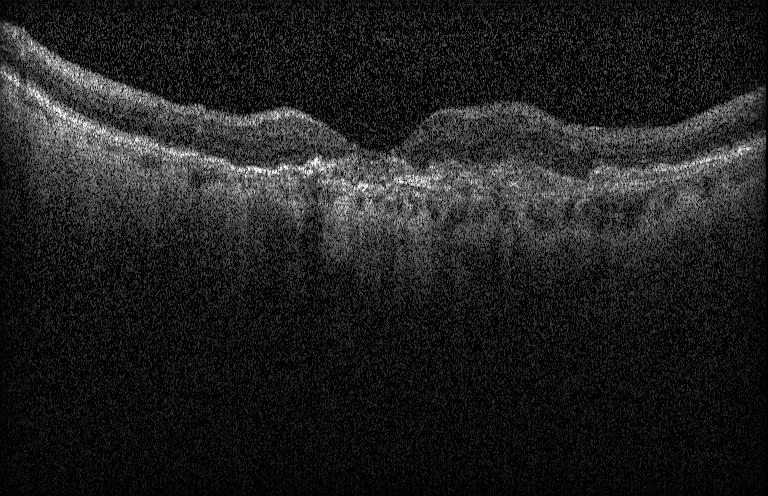 Retinal OCT B-scan
This B-scan demonstrates a choroidal neovascular membrane.